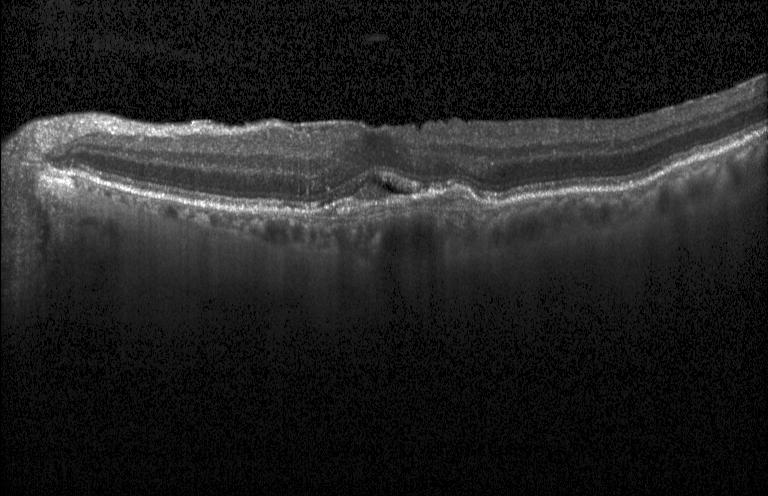

The scan shows choroidal neovascularization (CNV).